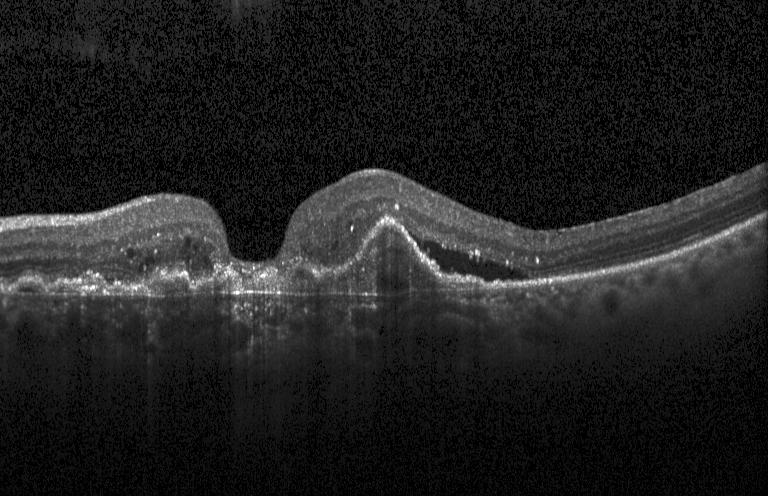 Spectral-domain OCT B-scan: CNV.